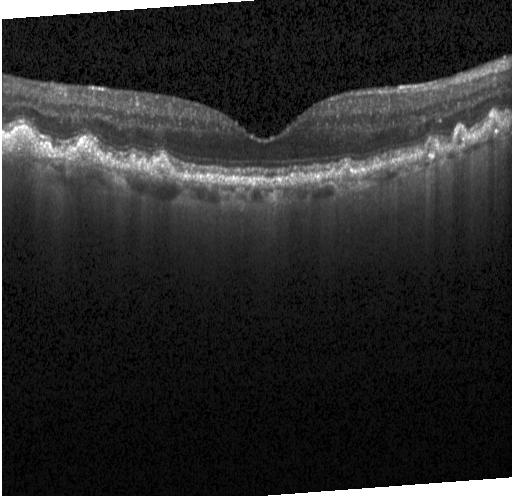 Assessment: drusen.